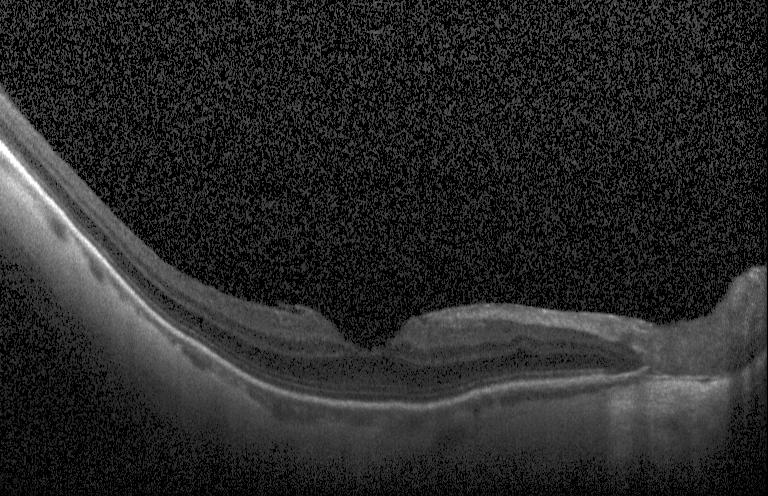

Impression: neither CNV, DME, nor drusen.